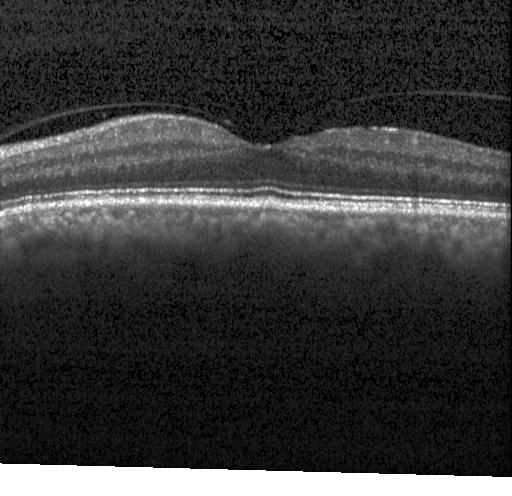
OCT B-scan showing no choroidal neovascularization, no diabetic macular edema, and no drusen.